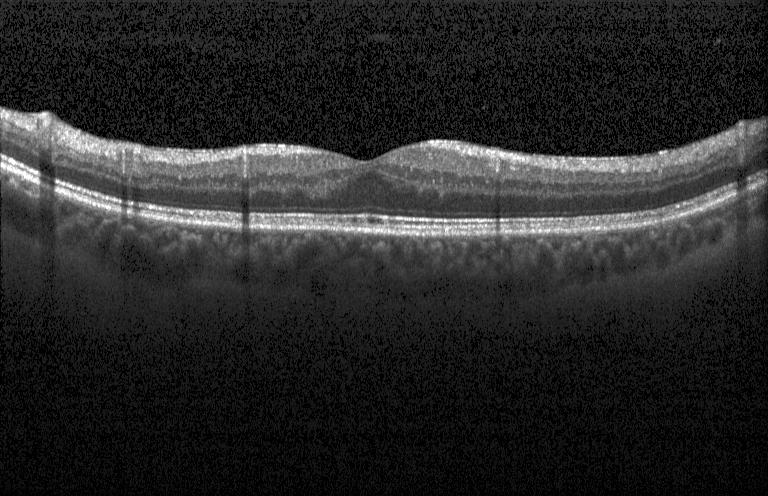 OCT B-scan showing no CNV, DME, or drusen.